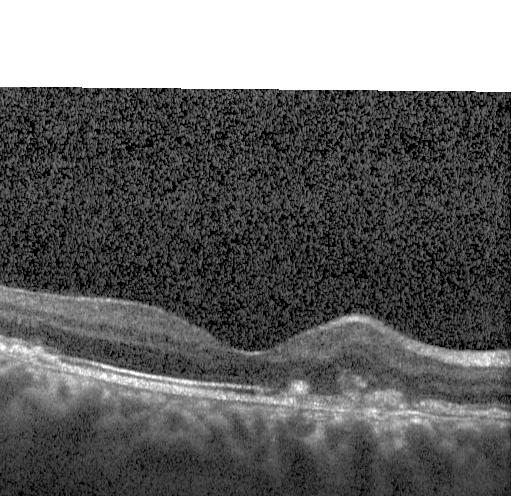

Through the macula. SD-OCT. Heidelberg Spectralis OCT system. Optical coherence tomography scan. Dx: a choroidal neovascular membrane.